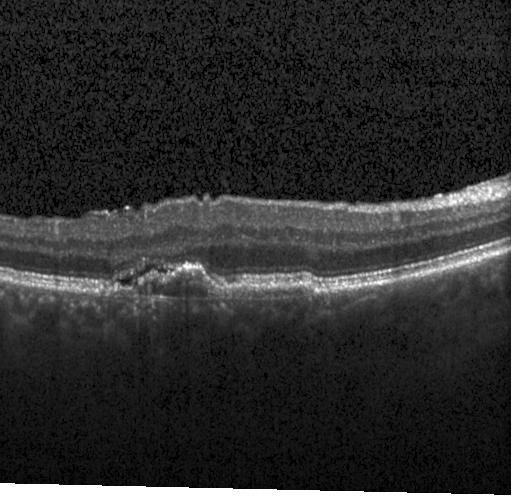
Spectral-domain optical coherence tomography; OCT line scan; acquired on a Heidelberg Spectralis.
Assessment: a choroidal neovascular membrane.